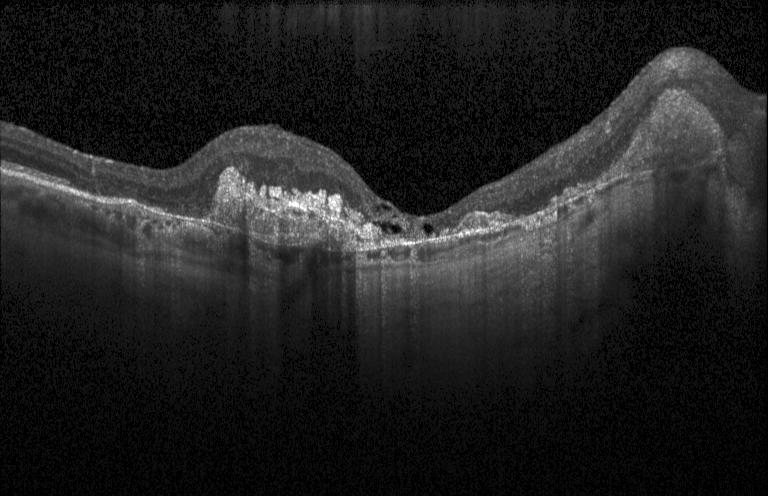

Impression: choroidal neovascularization.